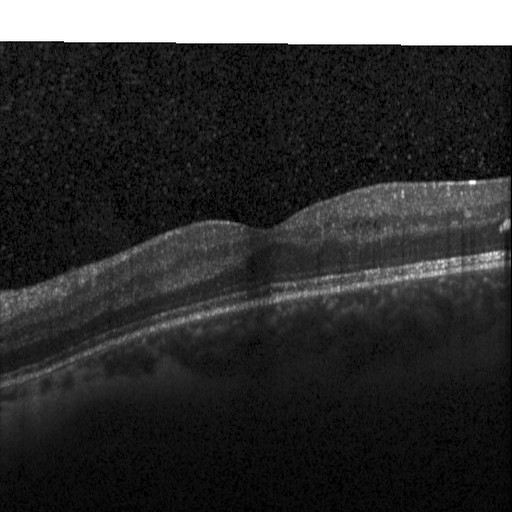
Optical coherence tomography B-scan, spectral-domain optical coherence tomography, Heidelberg Spectralis OCT system. Diabetic macular edema (DME).